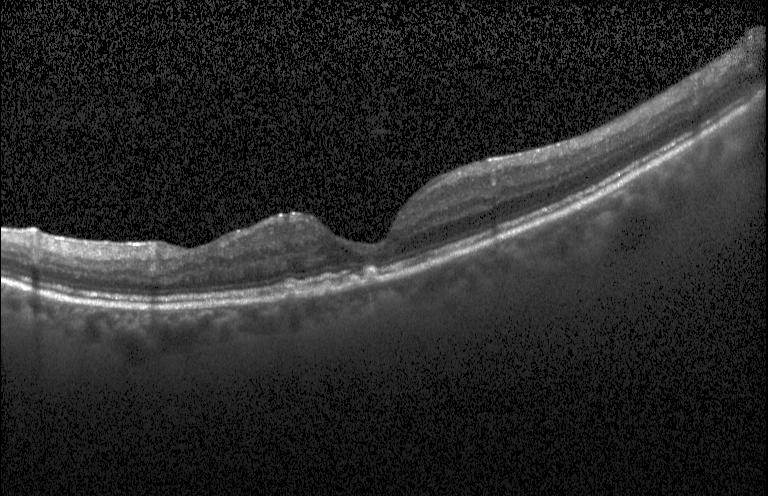 Diagnosis: multiple drusen.